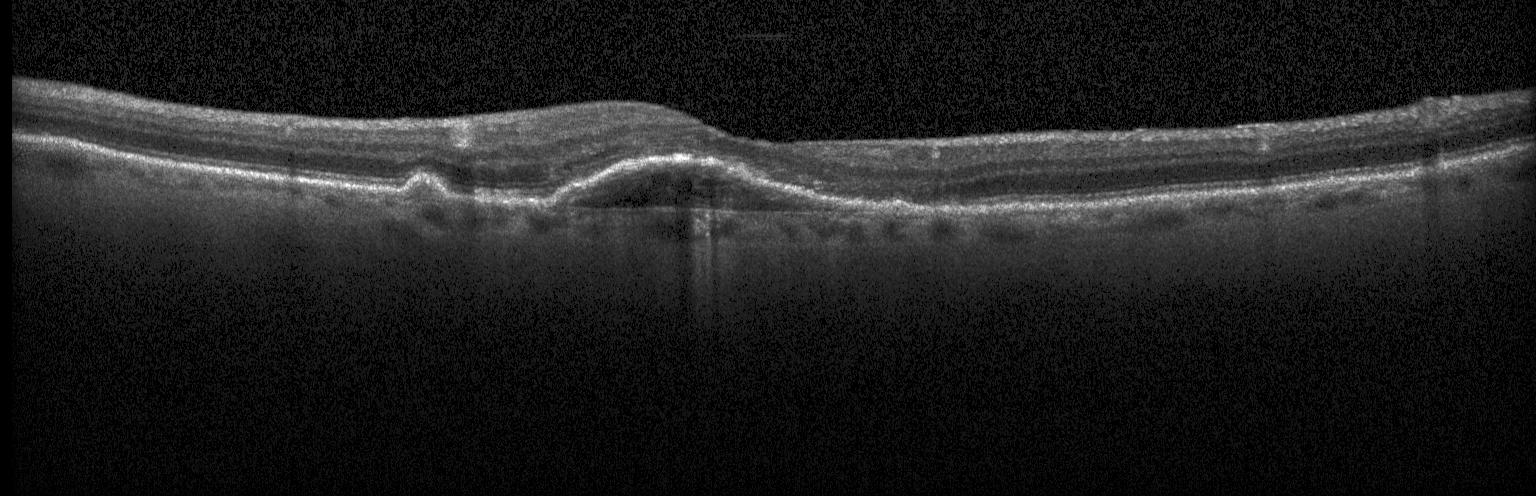
OCT line scan — Finding: a choroidal neovascular membrane.